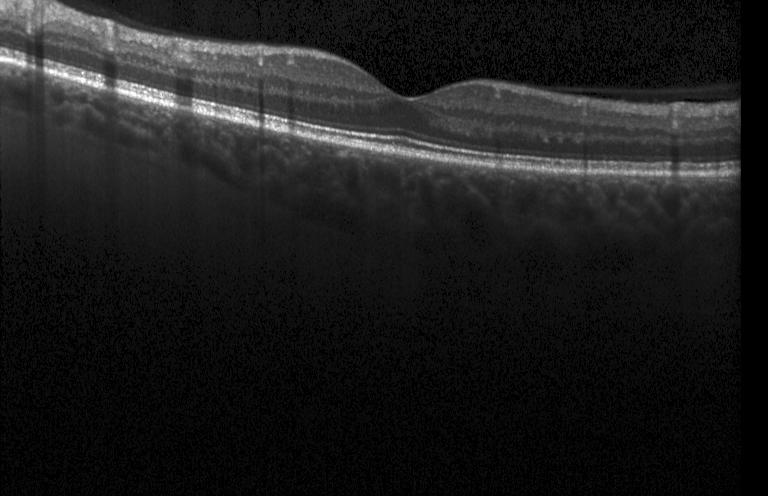

Spectral-domain OCT B-scan: no choroidal neovascularization, no diabetic macular edema, and no drusen.